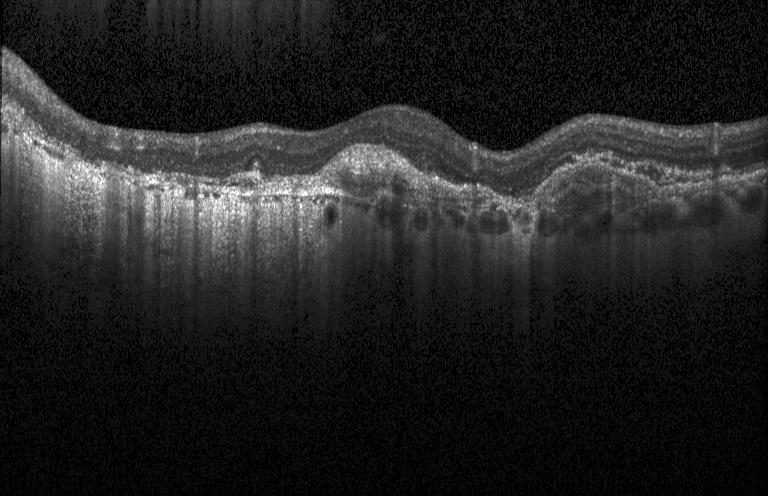
Impression: choroidal neovascularization (CNV).